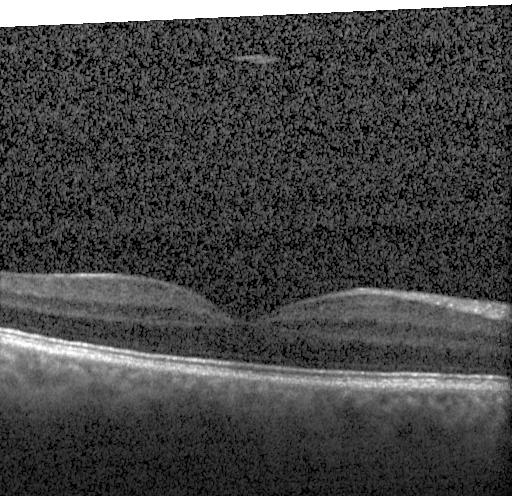

Spectral-domain optical coherence tomography; OCT B-scan
Impression: no choroidal neovascularization, diabetic macular edema, or drusen.